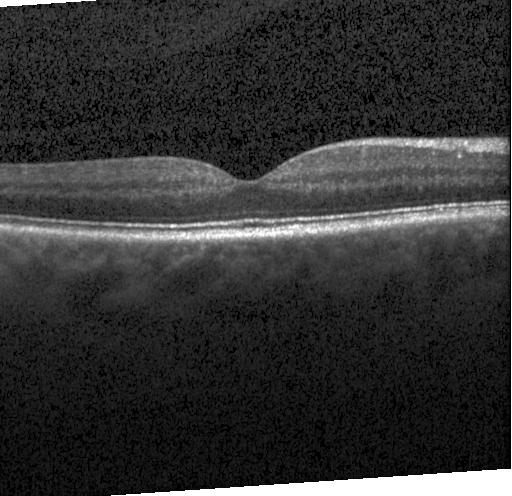

Impression: no choroidal neovascularization, diabetic macular edema, or drusen.